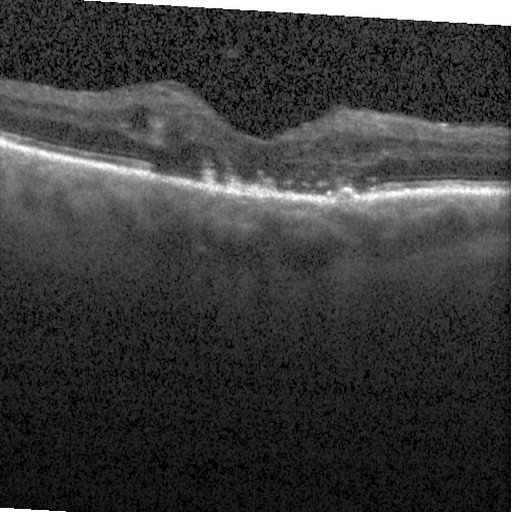

Impression: diabetic macular edema (DME).